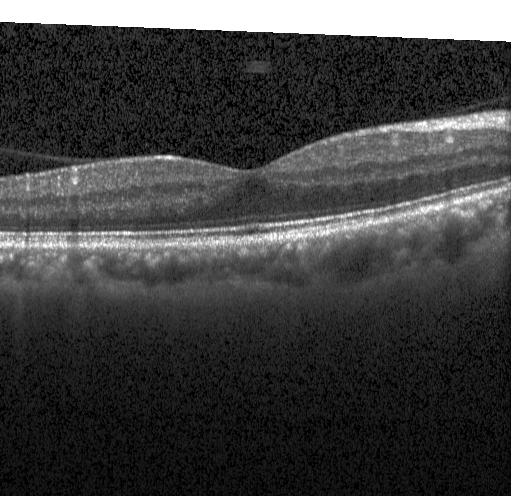
Through the macula. Retinal OCT cross-section
Impression: no evidence of CNV, DME, or drusen.